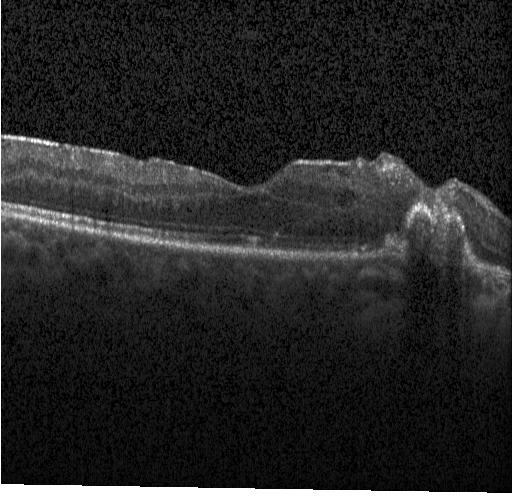 OCT B-scan
This B-scan demonstrates a choroidal neovascular membrane.